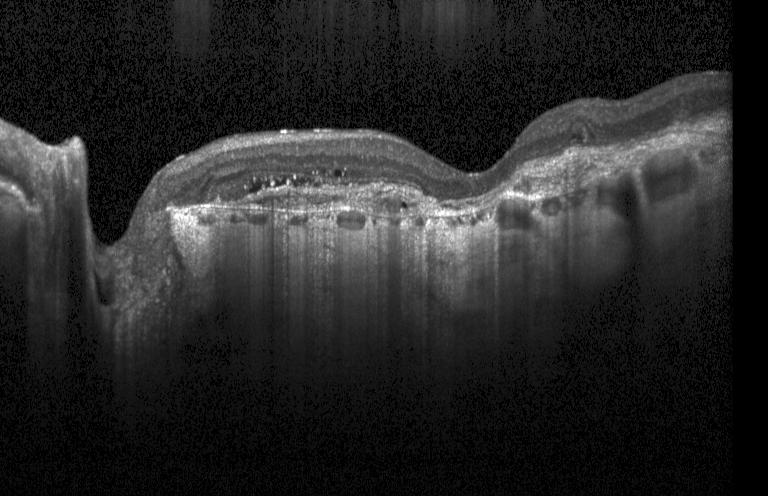

Impression: choroidal neovascularization.